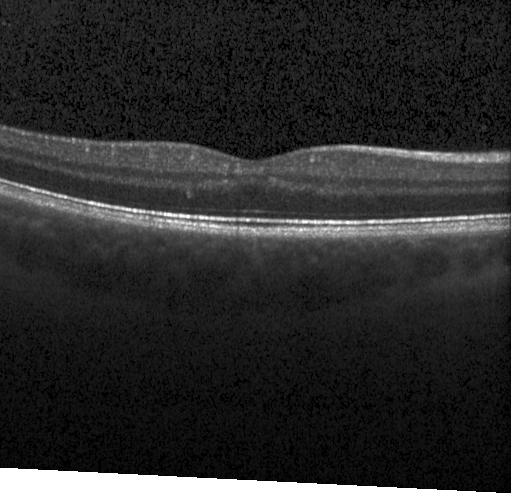

OCT line scan
Macular OCT: no choroidal neovascularization, no diabetic macular edema, and no drusen.